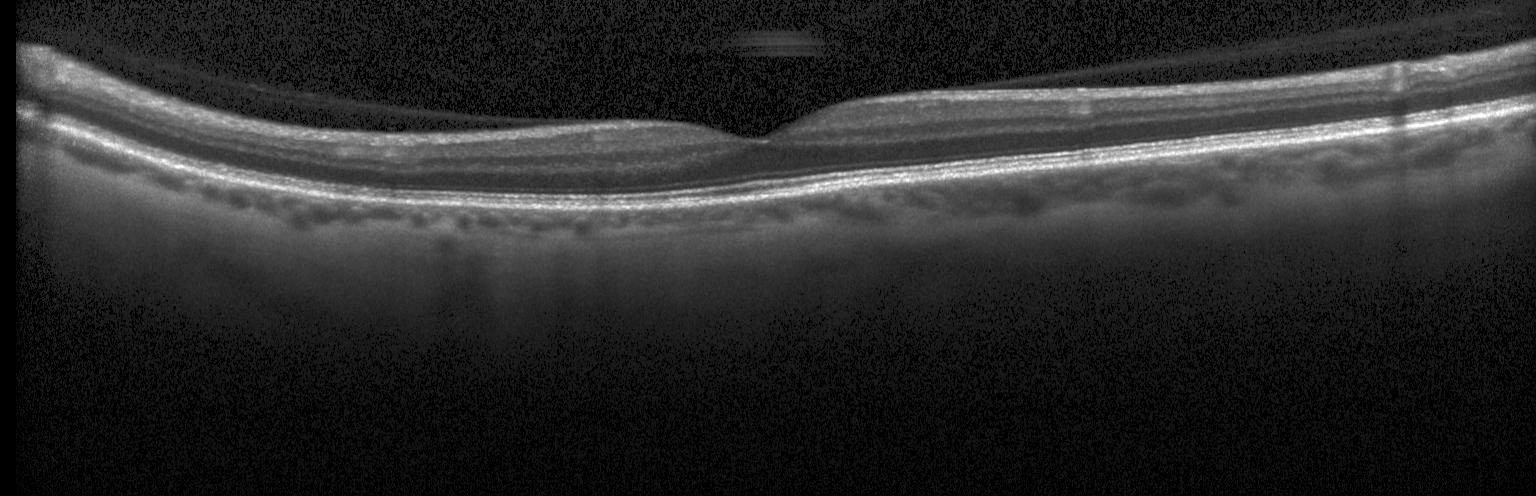
Spectral-domain OCT; acquired on a Heidelberg Spectralis; OCT line scan. Diagnosis: neither choroidal neovascularization, diabetic macular edema, nor drusen.